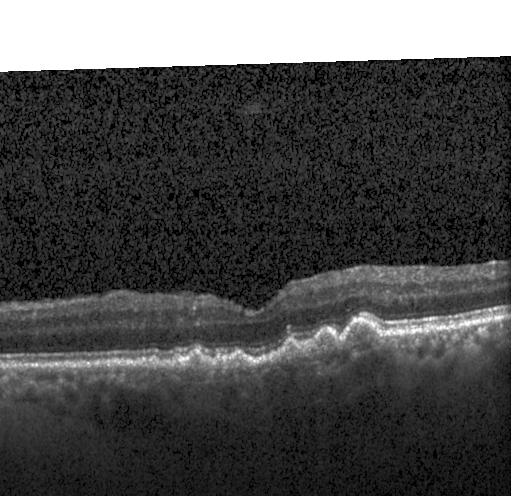
Instrument: Heidelberg Spectralis, retinal OCT cross-section
Assessment: sub-RPE drusenoid deposits.